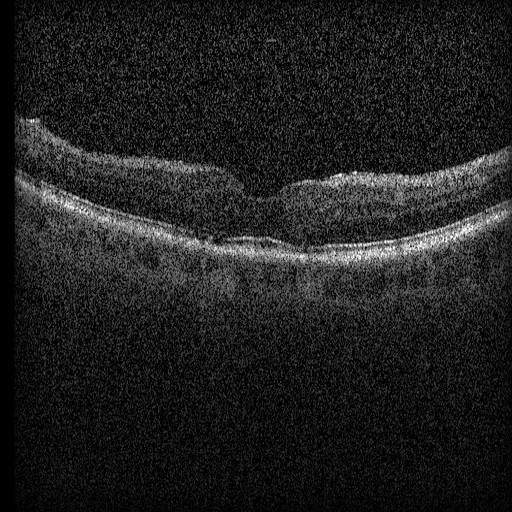 Macular OCT demonstrating diabetic macular edema.